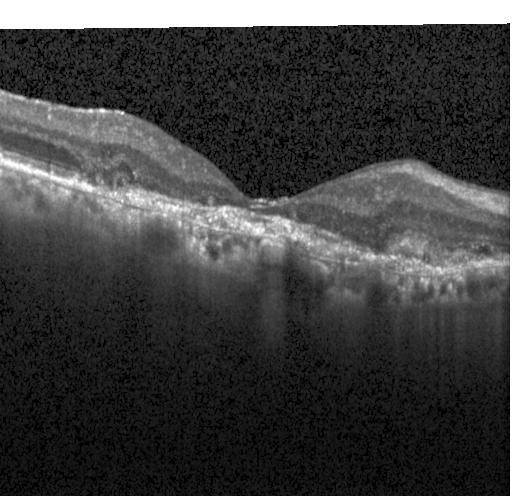 Optical coherence tomography scan — Diagnosis: a choroidal neovascular membrane.